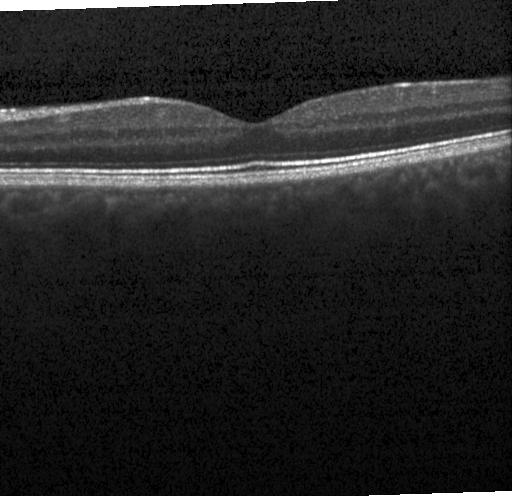 Retinal OCT B-scan.
Macular OCT: no CNV, DME, or drusen.